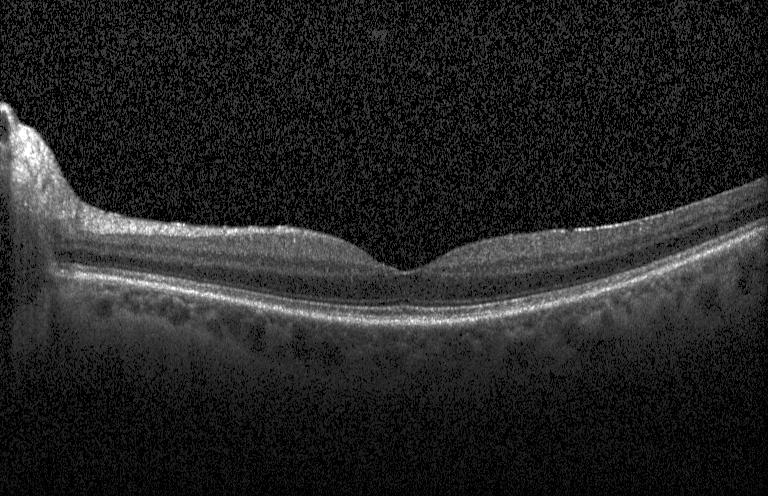 OCT finding: no choroidal neovascularization, diabetic macular edema, or drusen.